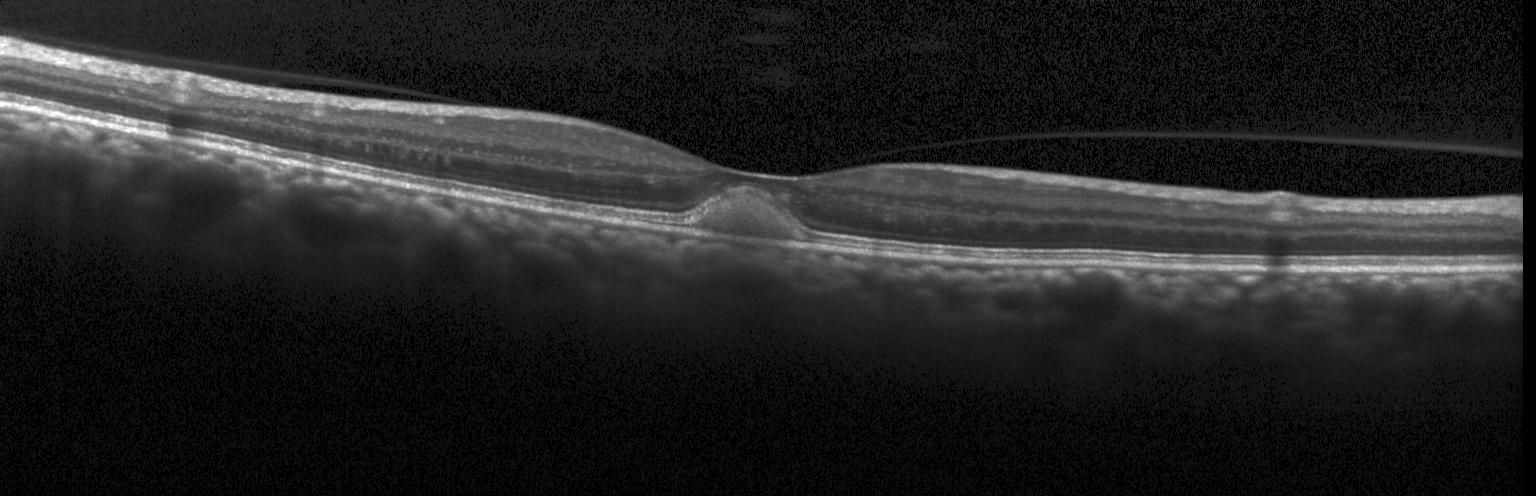

Heidelberg Spectralis. SD-OCT. Centered on the fovea. Optical coherence tomography B-scan. OCT finding: CNV.